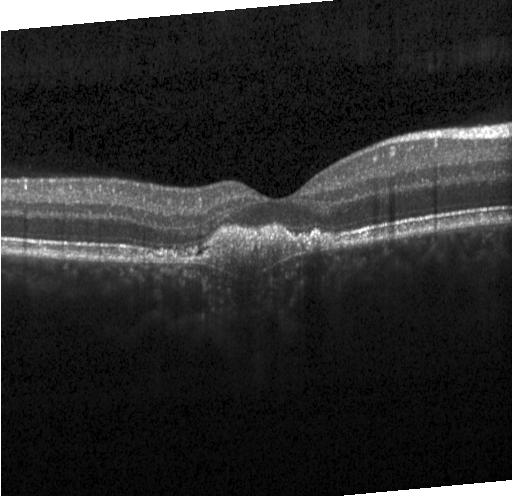

Assessment: CNV.